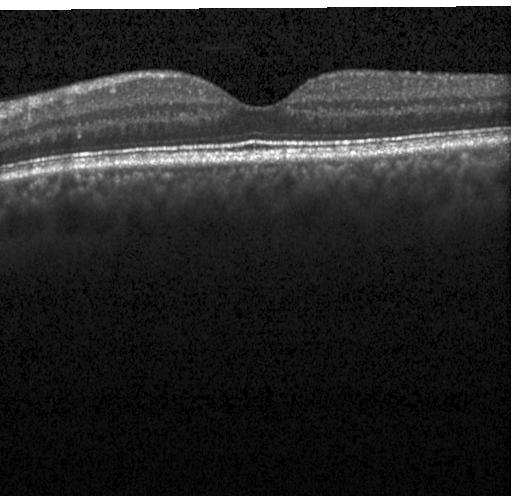 OCT line scan; Heidelberg Spectralis; through the macula
OCT finding: no evidence of CNV, DME, or drusen.